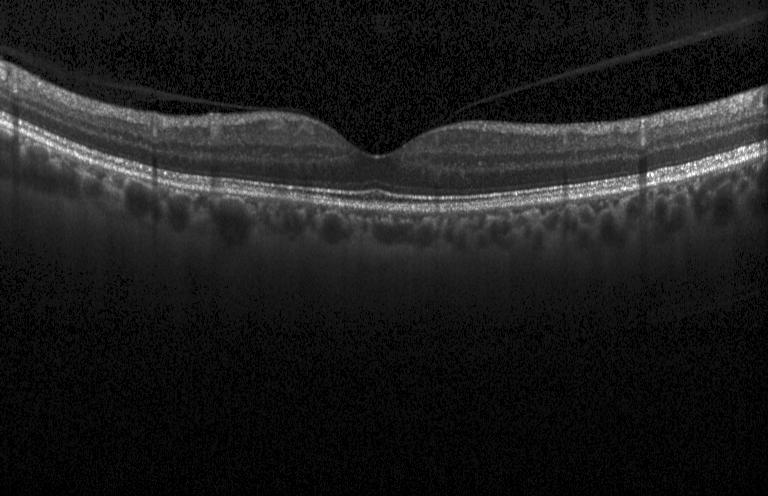 Macular OCT demonstrating neither choroidal neovascularization, diabetic macular edema, nor drusen.